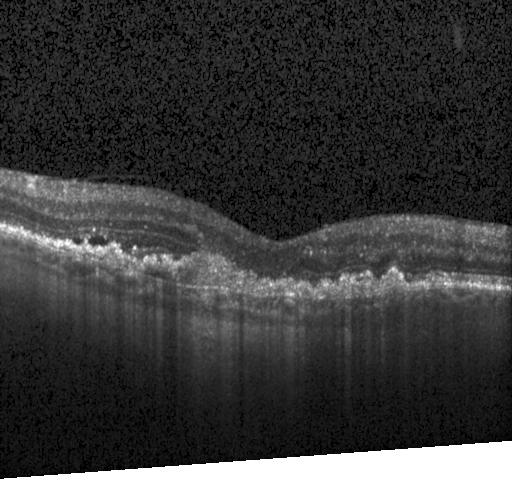 Spectral-domain OCT, optical coherence tomography scan. Impression: a choroidal neovascular membrane.